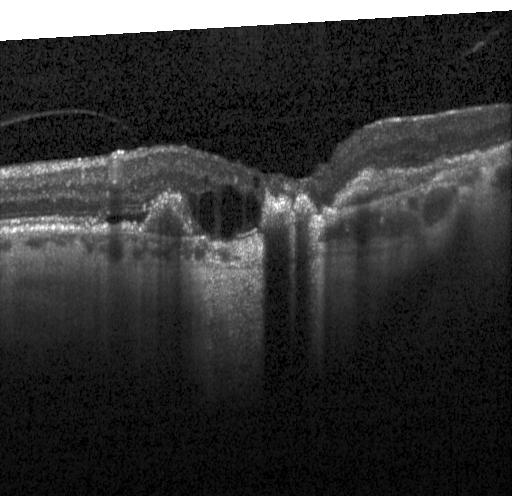

Retinal OCT B-scan. Horizontal scan through the fovea. Finding: choroidal neovascularization.